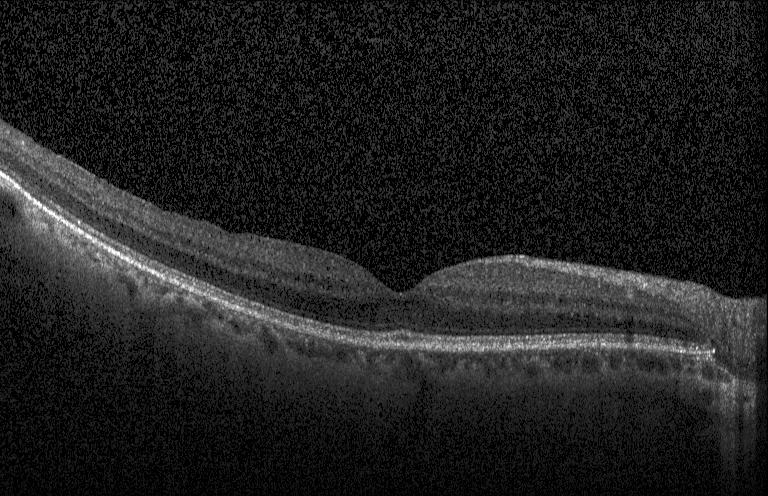
Retinal OCT B-scan. Finding: neither choroidal neovascularization, diabetic macular edema, nor drusen.